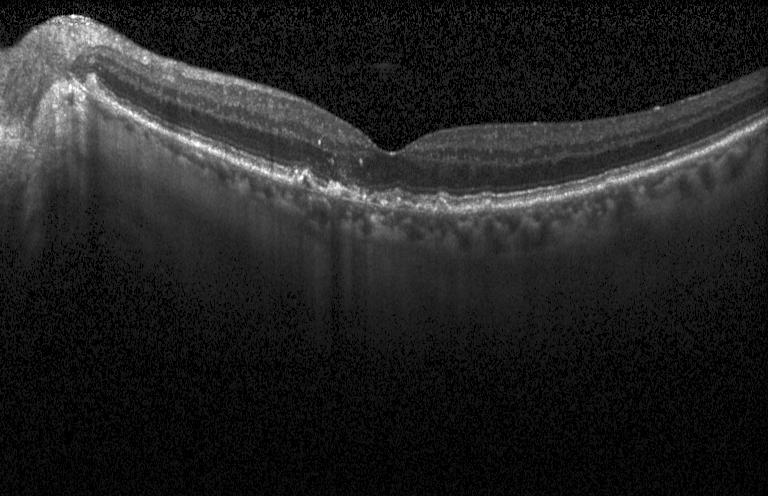

Finding: multiple drusen.